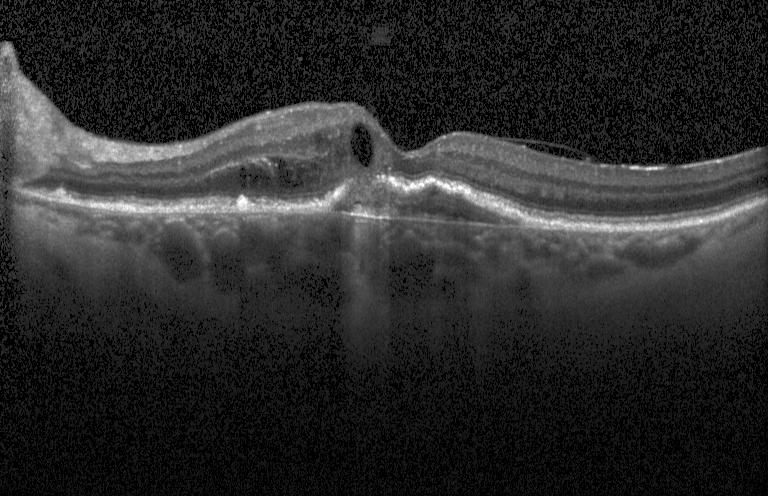
Optical coherence tomography scan. Acquired on a Heidelberg Spectralis. Horizontal scan through the fovea. Spectral-domain OCT. The scan shows CNV.